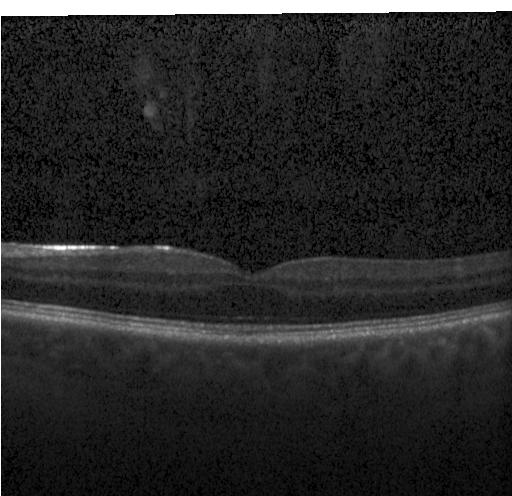
Optical coherence tomography B-scan — Diagnosis: no choroidal neovascularization, no diabetic macular edema, and no drusen.